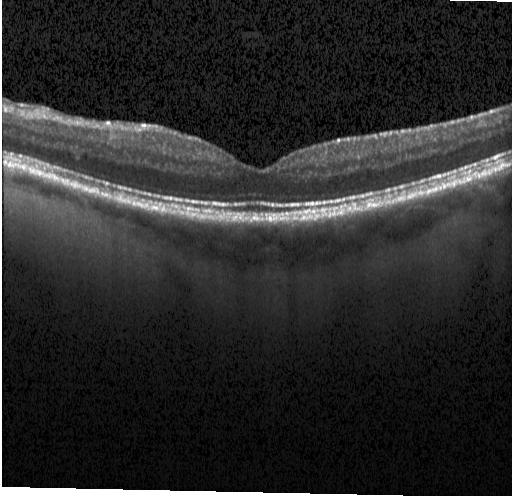

OCT B-scan. SD-OCT — Diagnosis: no evidence of choroidal neovascularization, diabetic macular edema, or drusen.